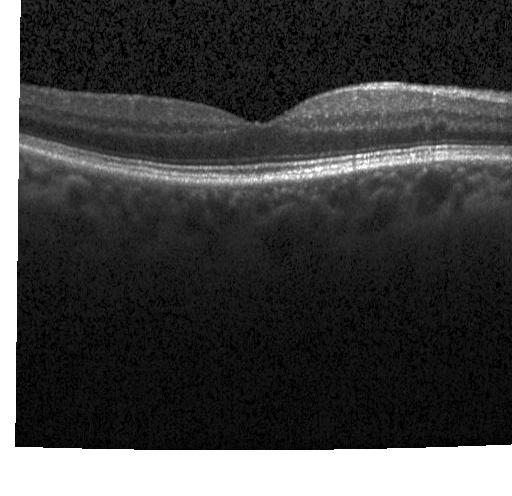
Heidelberg Spectralis; spectral-domain OCT; horizontal scan through the fovea; optical coherence tomography scan
Impression: neither choroidal neovascularization, diabetic macular edema, nor drusen.